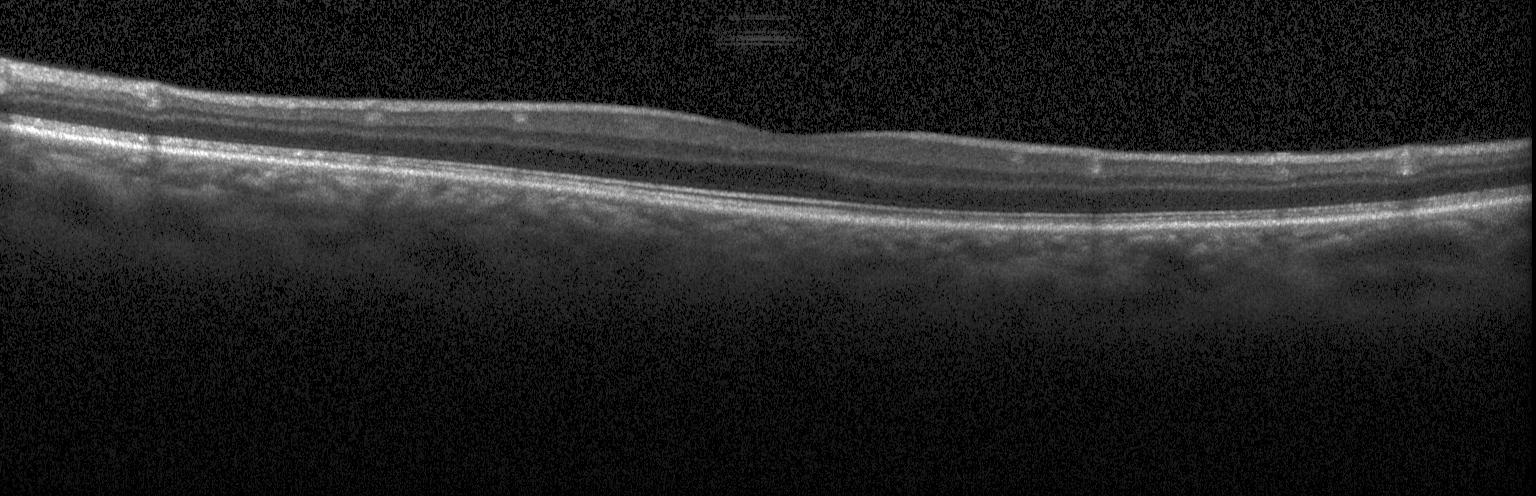

Spectral-domain OCT. Through the macula. Retinal OCT cross-section
Dx: no CNV, DME, or drusen.